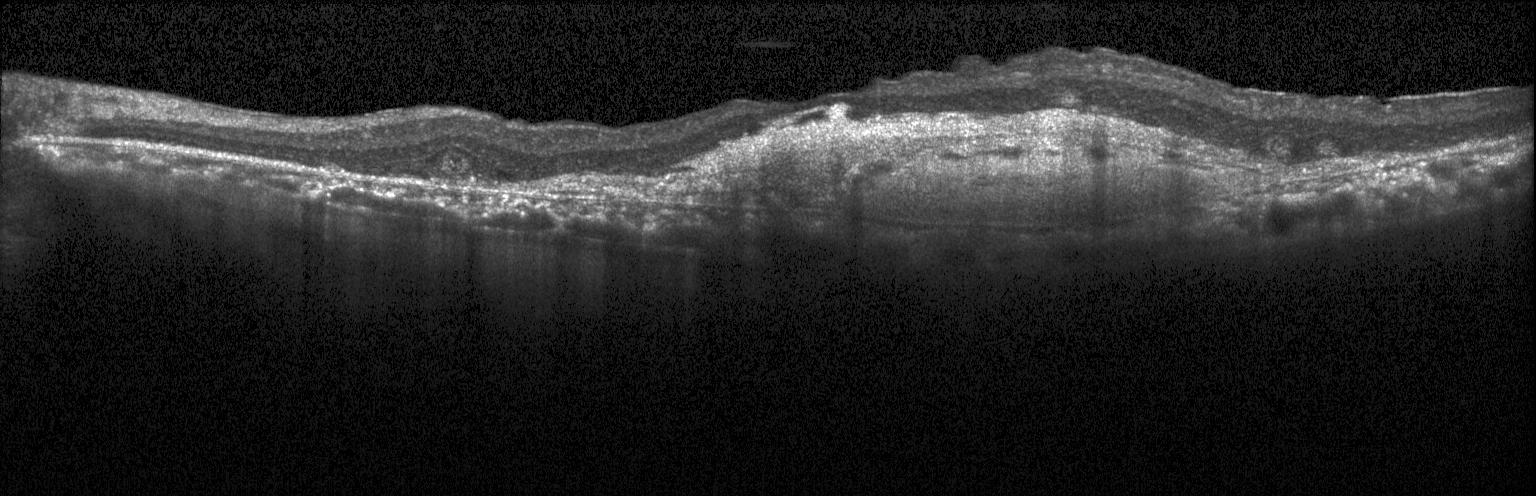

Retinal OCT cross-section showing a choroidal neovascular membrane.